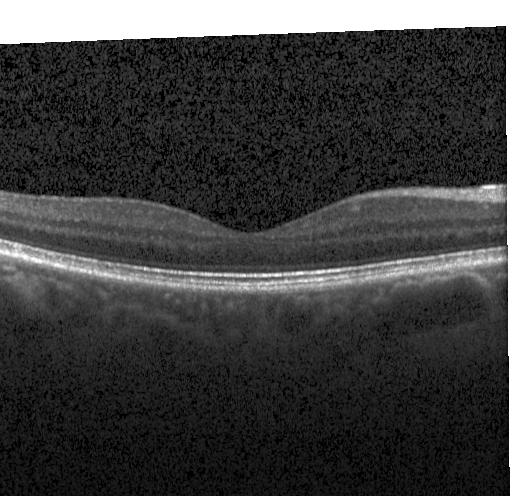 Optical coherence tomography B-scan.
This B-scan demonstrates no choroidal neovascularization, no diabetic macular edema, and no drusen.